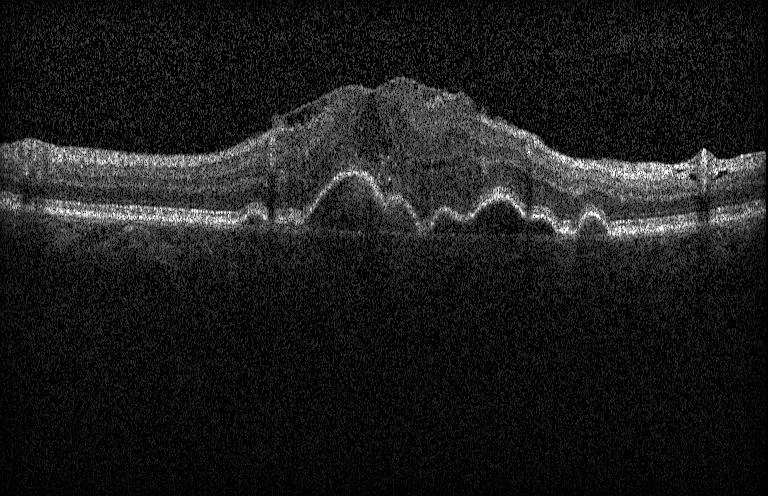
Macular scan. OCT line scan
Choroidal neovascularization (CNV).